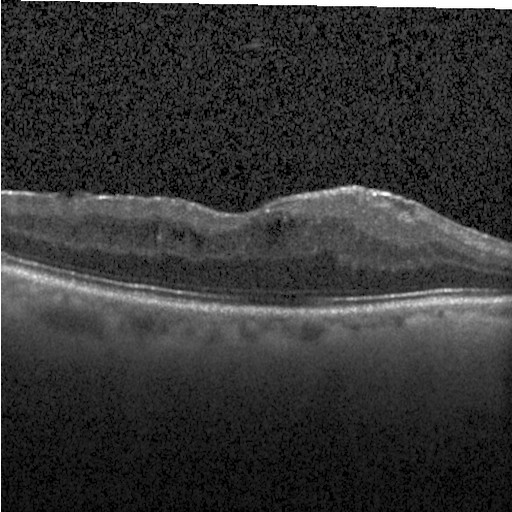
Diagnosis: diabetic macular edema (DME).